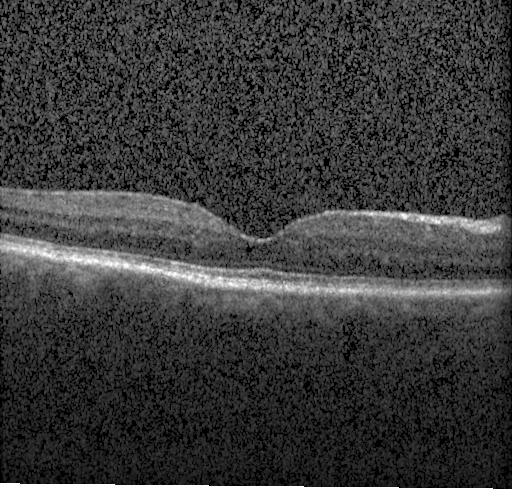
Macular OCT: no evidence of choroidal neovascularization, diabetic macular edema, or drusen.